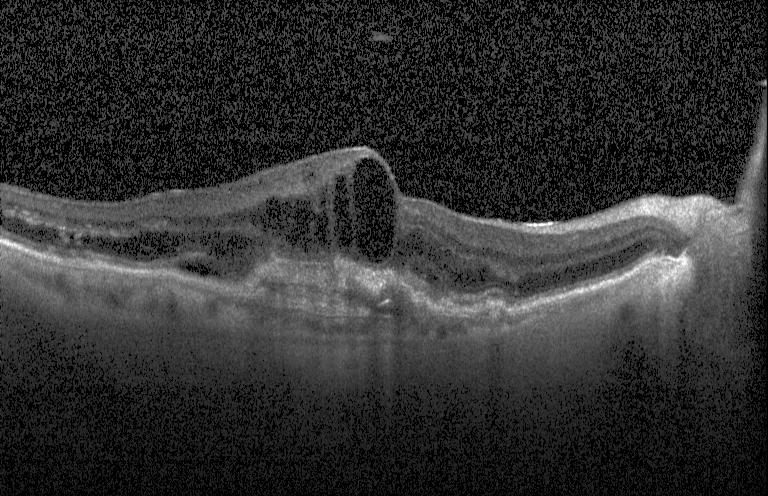 Optical coherence tomography B-scan · through the macula · Heidelberg Spectralis OCT system · SD-OCT
The scan shows choroidal neovascularization (CNV).